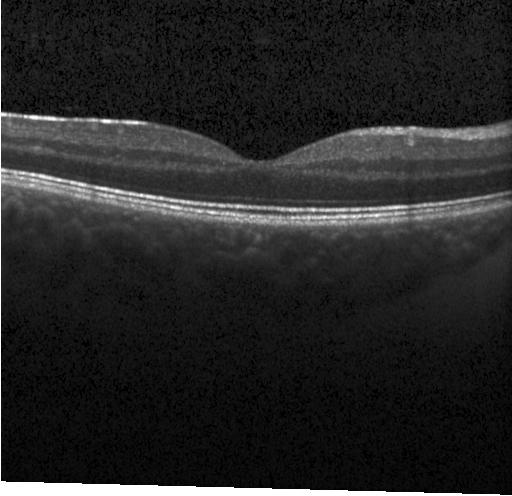 Instrument: Heidelberg Spectralis; centered on the fovea; OCT line scan. OCT finding: neither choroidal neovascularization, diabetic macular edema, nor drusen.